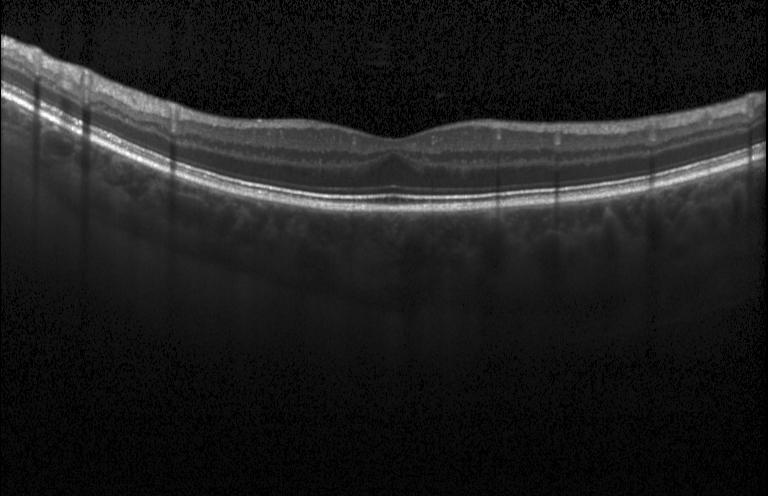 Fovea-centered. SD-OCT. Heidelberg Spectralis. Retinal OCT B-scan. This B-scan demonstrates neither choroidal neovascularization, diabetic macular edema, nor drusen.